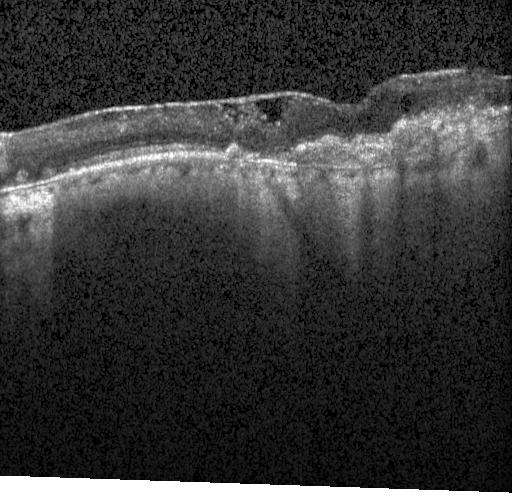 Instrument: Heidelberg Spectralis · spectral-domain OCT · OCT B-scan.
Finding: CNV.